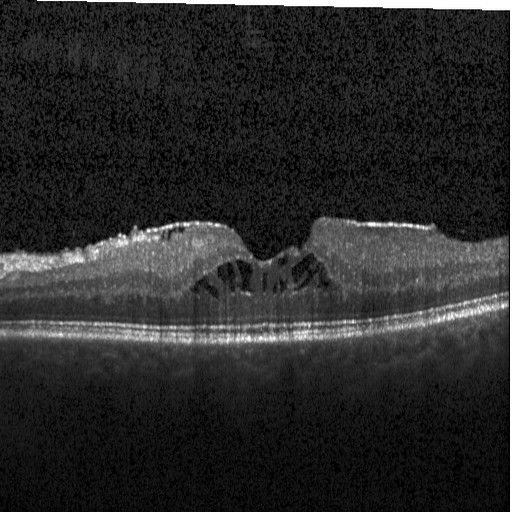 Retinal OCT B-scan
Diagnosis: diabetic macular edema (DME).